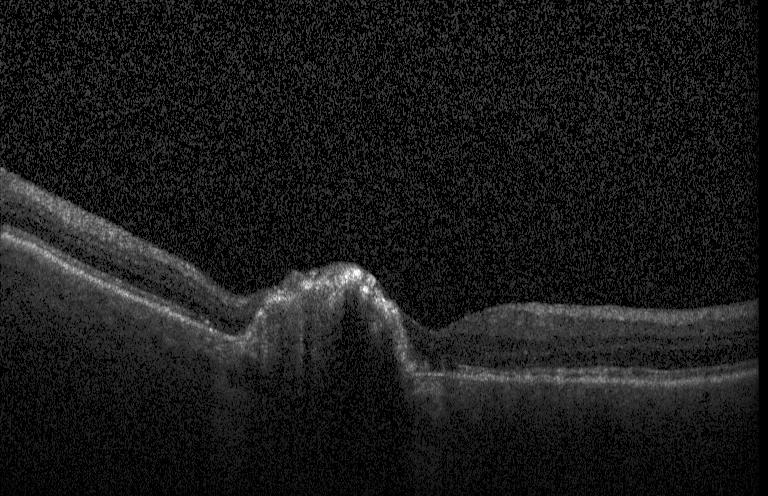

Spectral-domain optical coherence tomography · fovea-centered · OCT B-scan. Diagnosis: a choroidal neovascular membrane.